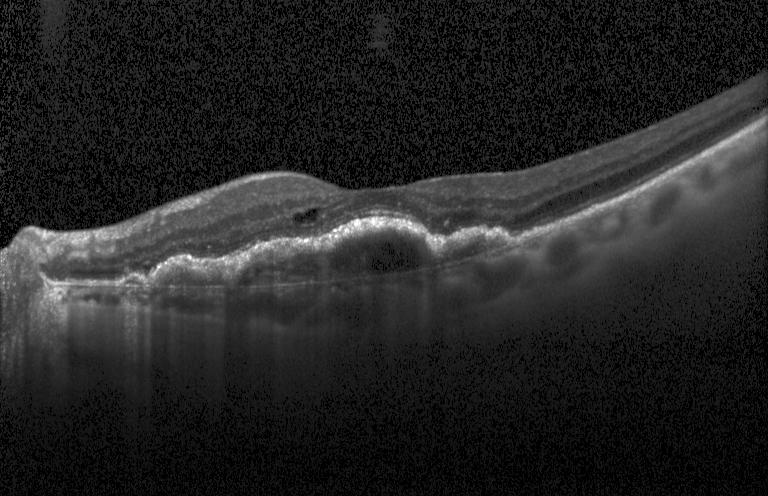 OCT B-scan; spectral-domain OCT; Heidelberg Spectralis; fovea-centered — Finding: CNV.